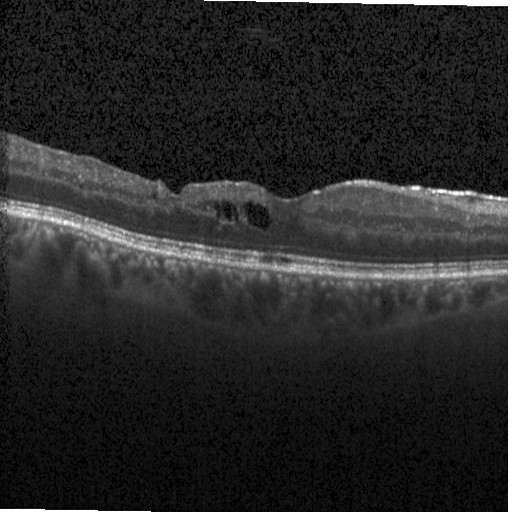 Instrument: Heidelberg Spectralis, OCT B-scan, spectral-domain optical coherence tomography, through the macula. This B-scan demonstrates diabetic macular edema.